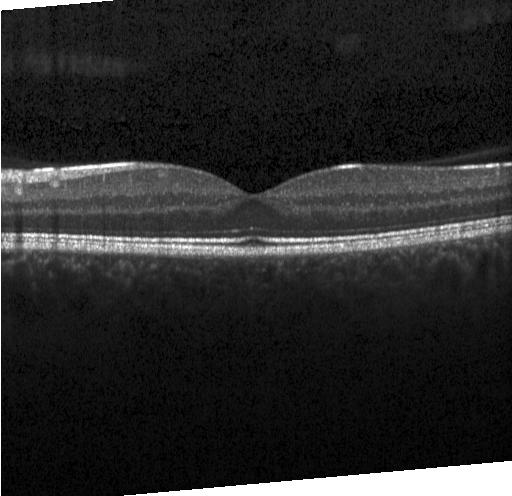
OCT scan showing neither choroidal neovascularization, diabetic macular edema, nor drusen.